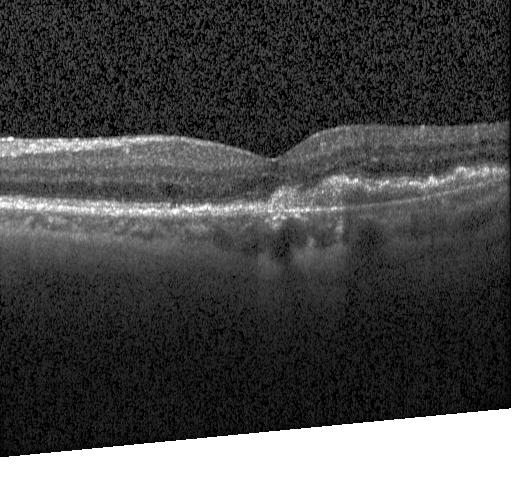

Through the macula, optical coherence tomography scan
Diagnosis: choroidal neovascularization (CNV).